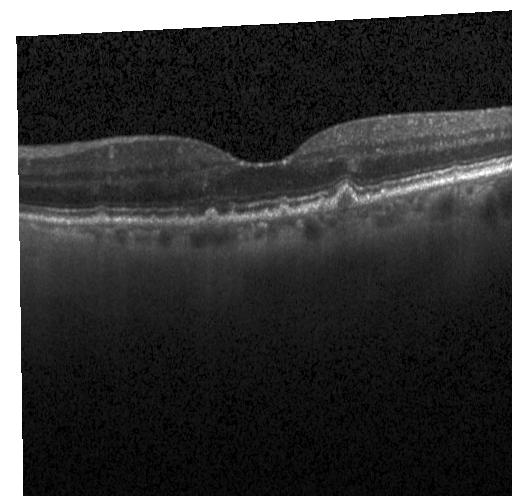
Finding: drusen.